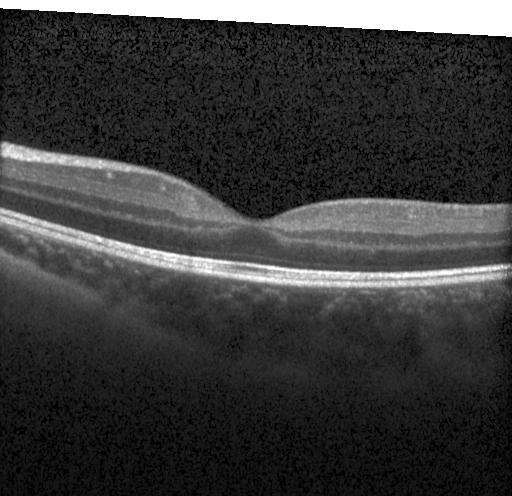 Retinal OCT cross-section showing no CNV, DME, or drusen.